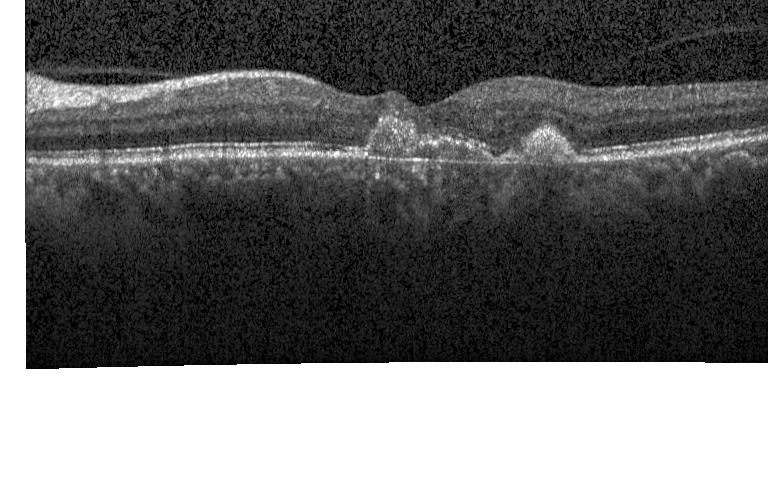 Diagnosis: choroidal neovascularization (CNV).